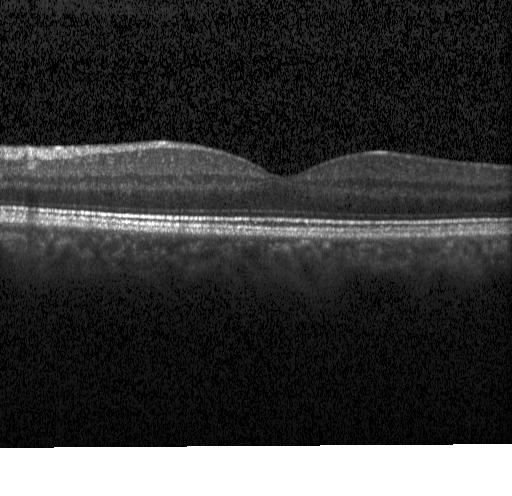 Optical coherence tomography scan — Diagnosis: neither CNV, DME, nor drusen.